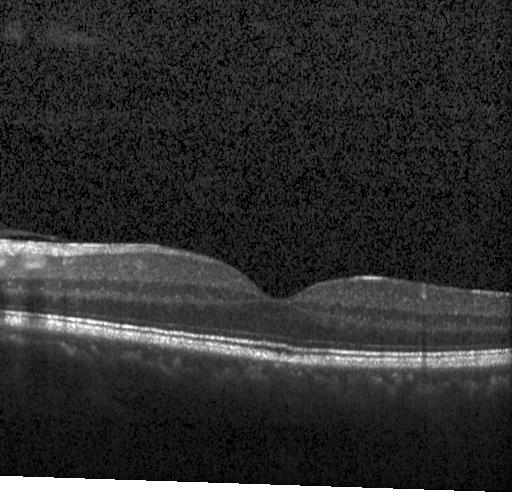 Assessment: no evidence of CNV, DME, or drusen.